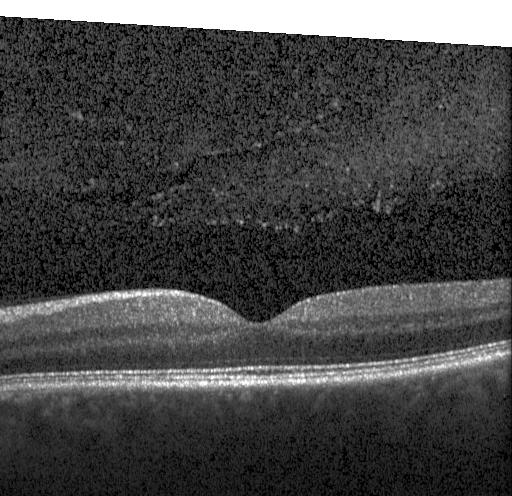

Retinal OCT cross-section showing no evidence of CNV, DME, or drusen.